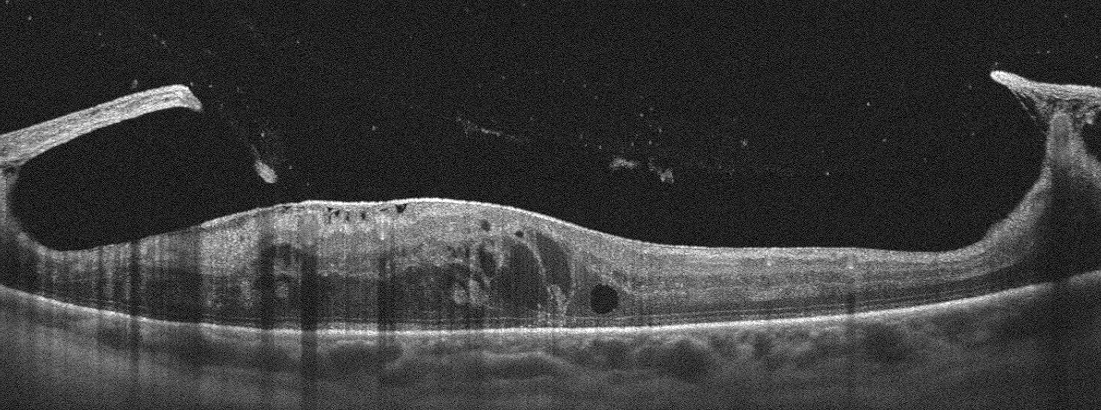
Impression: DME.